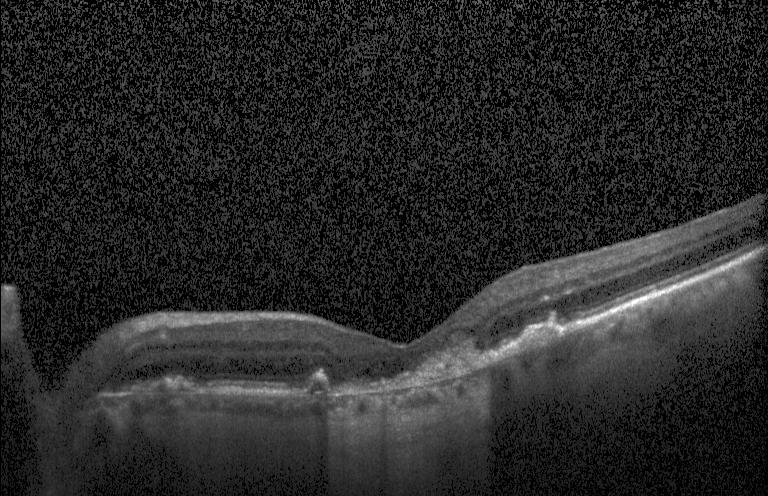
Retinal OCT B-scan — Macular OCT: a choroidal neovascular membrane.